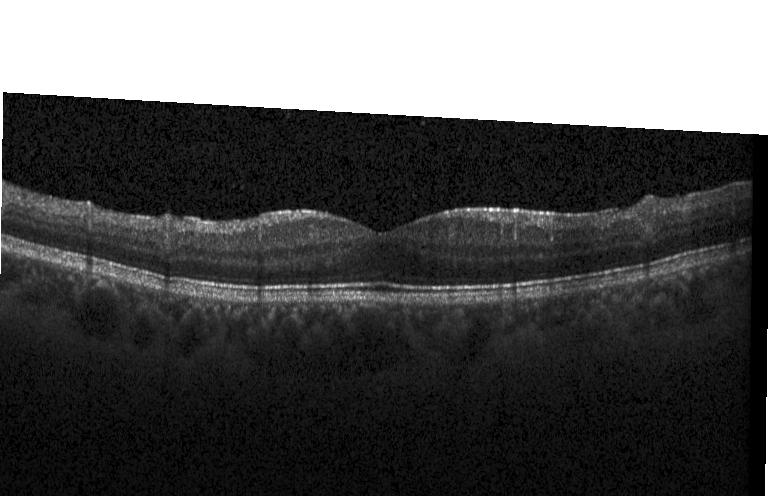

Impression: no choroidal neovascularization, diabetic macular edema, or drusen.